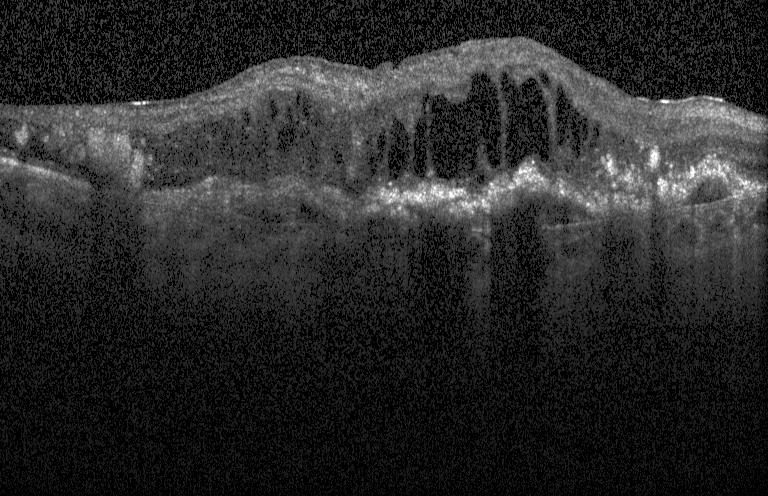 Fovea-centered; Heidelberg Spectralis OCT system; spectral-domain OCT; retinal OCT B-scan
Diagnosis: a choroidal neovascular membrane.